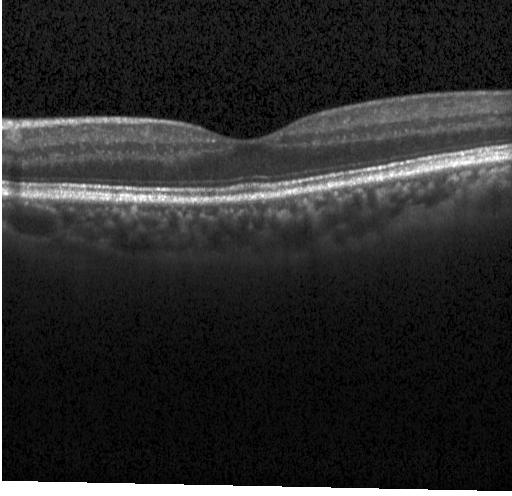

Finding: no choroidal neovascularization, diabetic macular edema, or drusen.